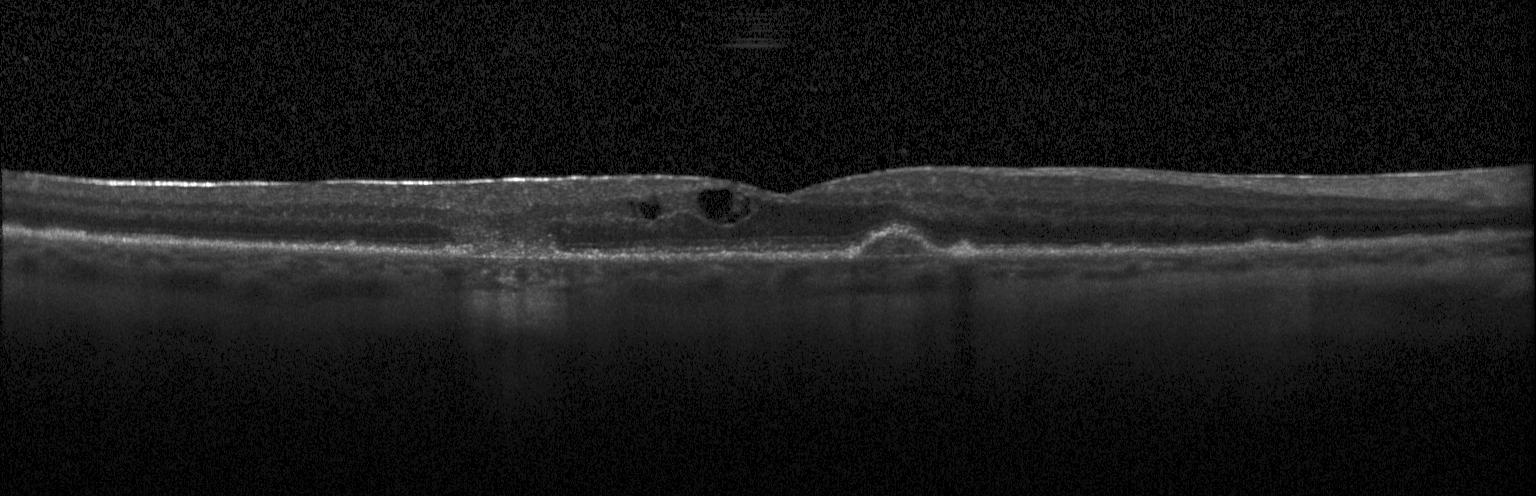 Impression: a choroidal neovascular membrane.